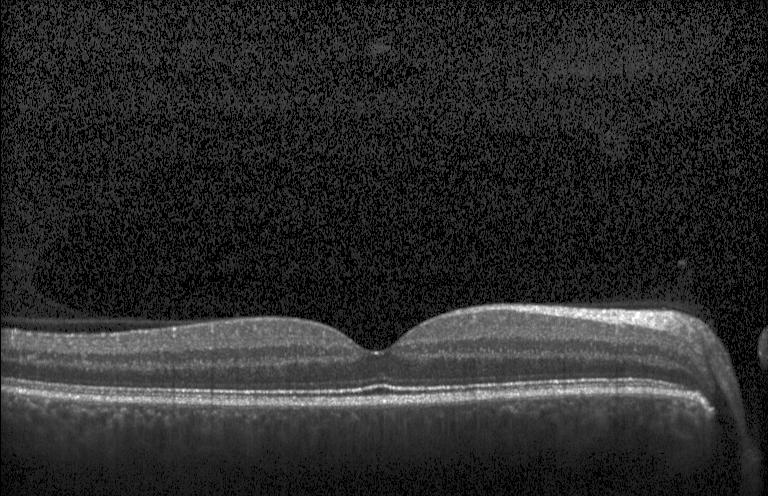

Spectral-domain OCT; optical coherence tomography scan; macular scan.
Assessment: neither CNV, DME, nor drusen.